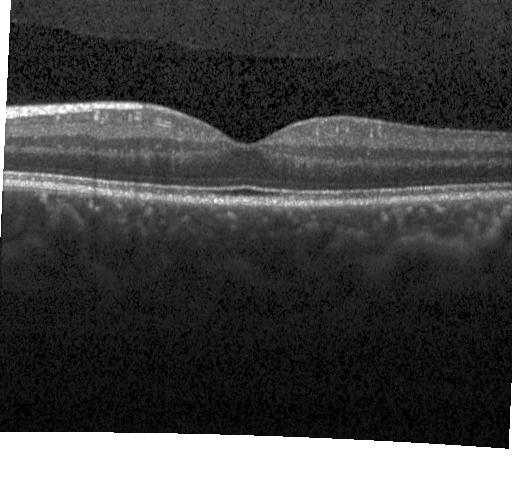
Heidelberg Spectralis OCT system · retinal OCT cross-section · spectral-domain OCT — Dx: no choroidal neovascularization, diabetic macular edema, or drusen.